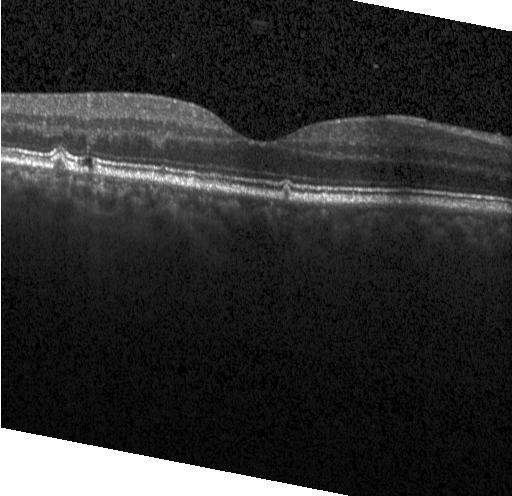
Diagnosis: drusen.